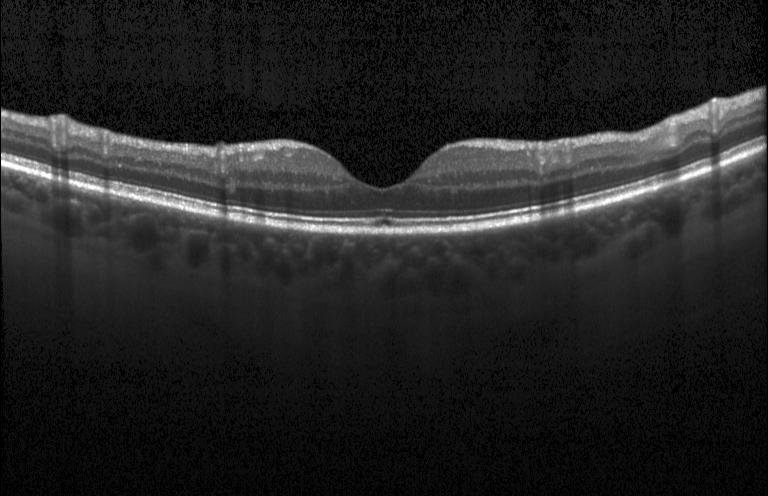 Retinal OCT cross-section showing no evidence of choroidal neovascularization, diabetic macular edema, or drusen.